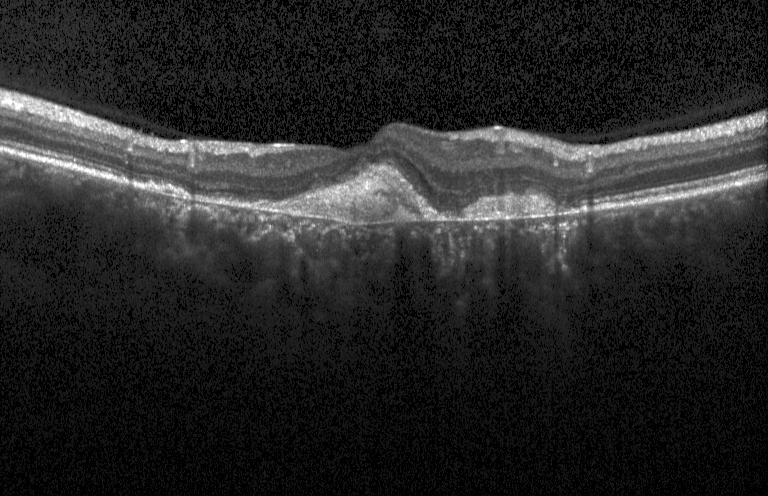 Instrument: Heidelberg Spectralis · OCT B-scan.
A choroidal neovascular membrane.